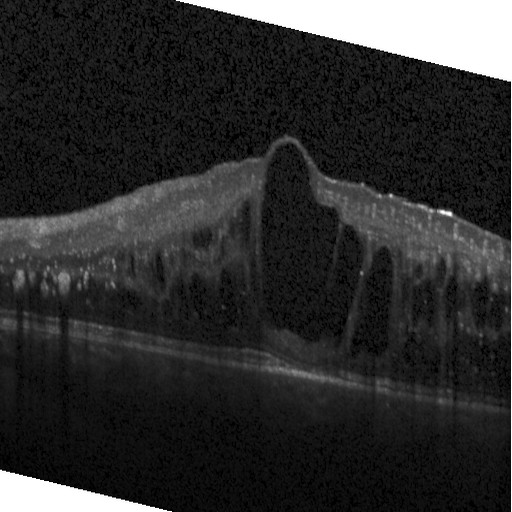
Horizontal scan through the fovea; OCT B-scan.
Macular OCT: diabetic macular edema.